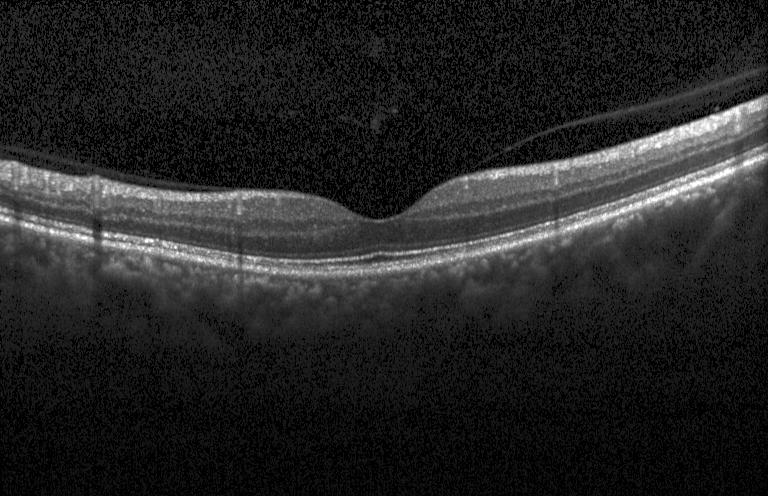

Impression: no CNV, DME, or drusen.